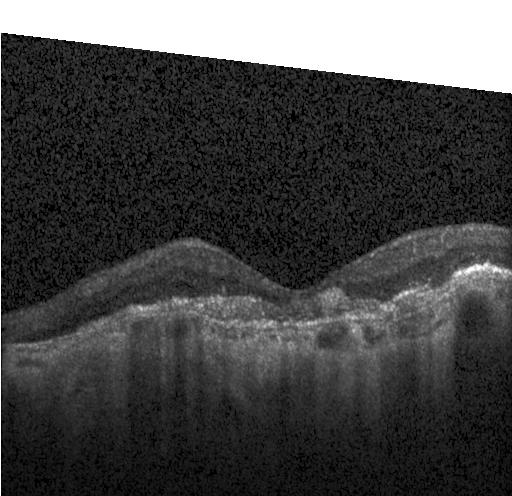
Impression: CNV.